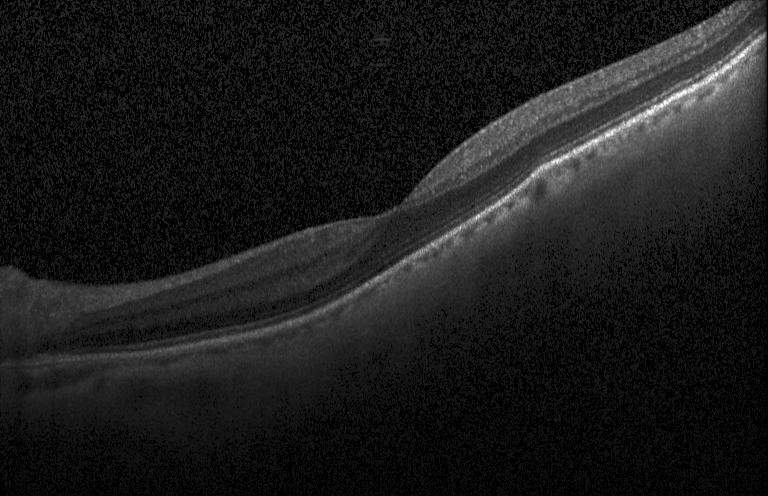 Heidelberg Spectralis OCT system; spectral-domain optical coherence tomography; OCT line scan
OCT finding: neither choroidal neovascularization, diabetic macular edema, nor drusen.